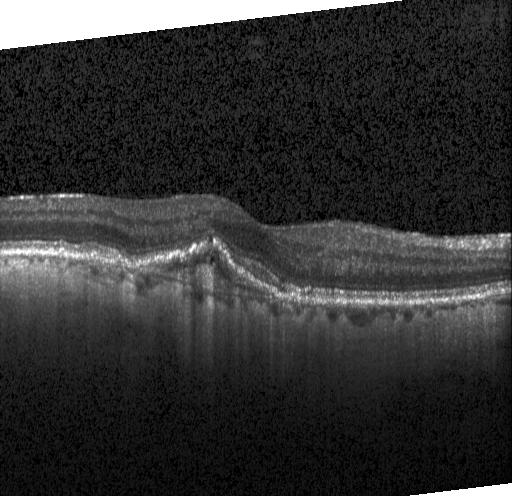 Macular OCT: CNV.